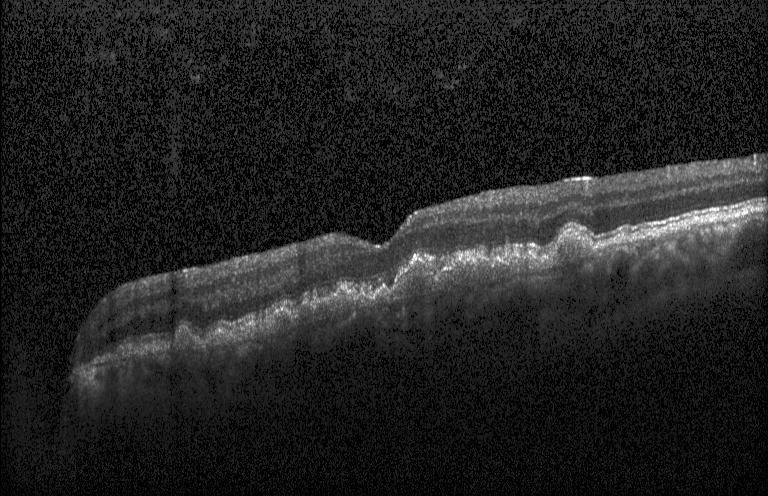
OCT line scan.
Finding: choroidal neovascularization.